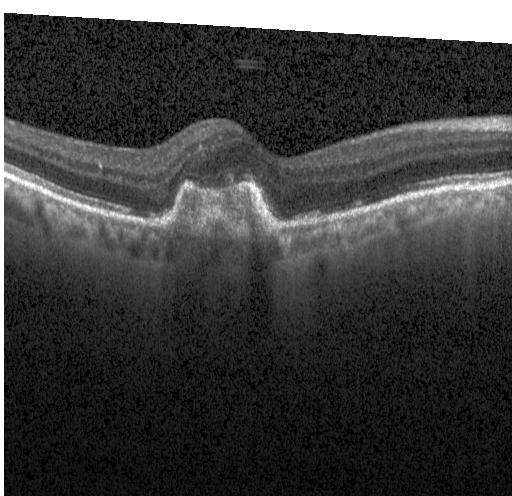 This B-scan demonstrates a choroidal neovascular membrane.